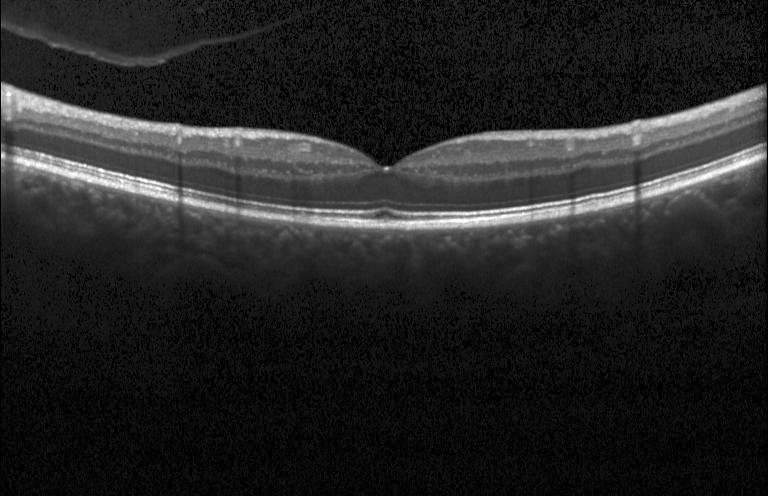

Optical coherence tomography scan. Impression: neither choroidal neovascularization, diabetic macular edema, nor drusen.